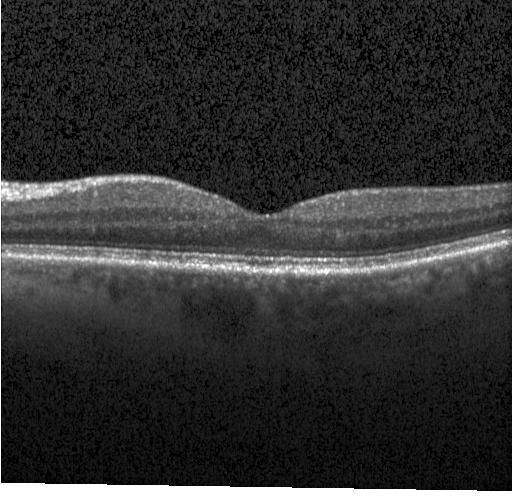
Diagnosis: no CNV, no DME, and no drusen.